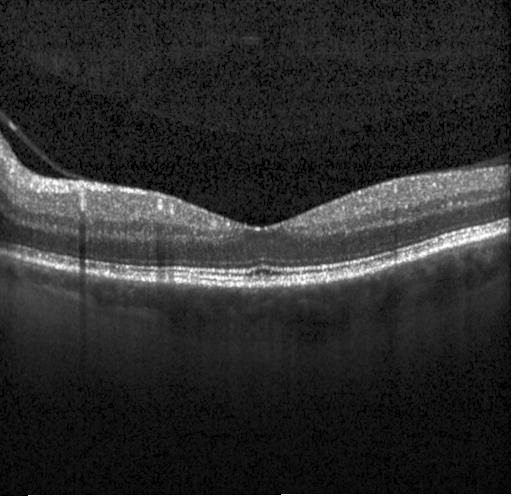
Optical coherence tomography scan
The scan shows no choroidal neovascularization, no diabetic macular edema, and no drusen.